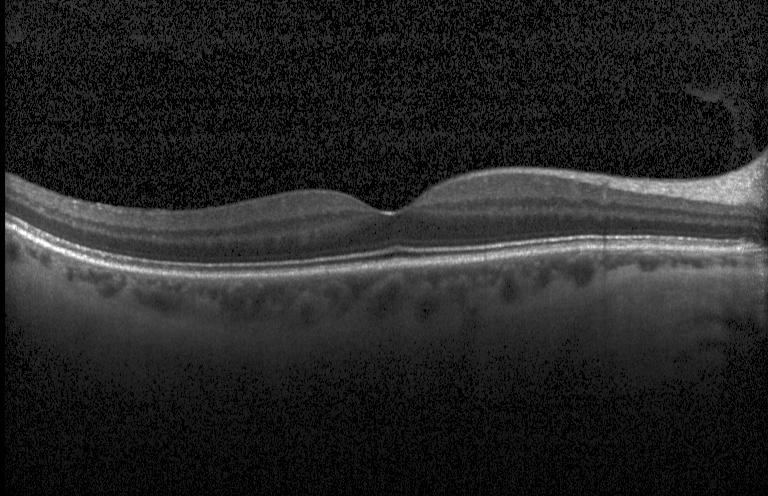
Diagnosis: no choroidal neovascularization, no diabetic macular edema, and no drusen.